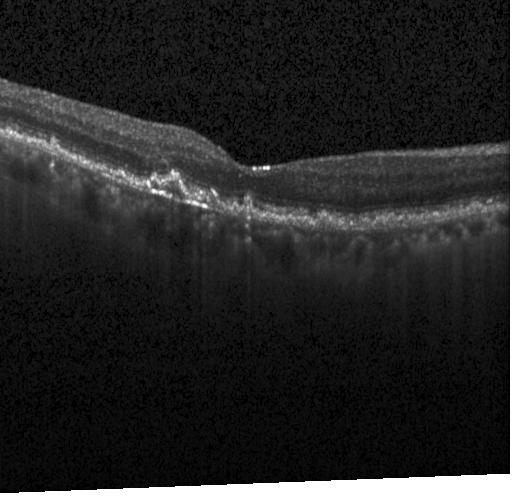 SD-OCT · optical coherence tomography B-scan · centered on the fovea
Macular OCT: choroidal neovascularization.